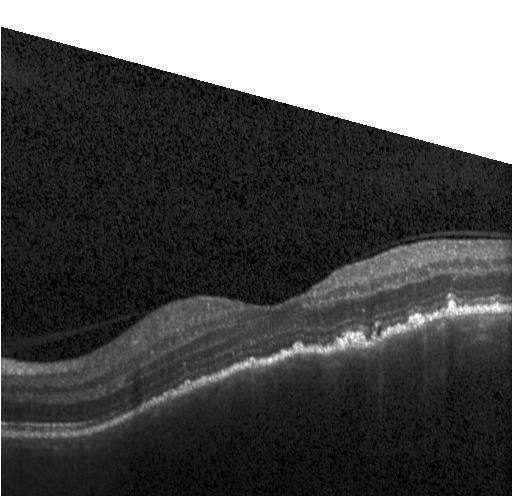

Optical coherence tomography scan · centered on the fovea — This B-scan demonstrates multiple drusen.